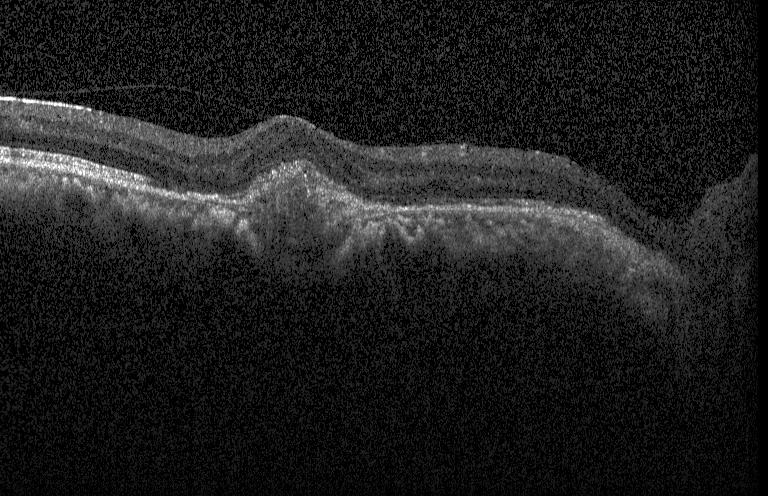

Diagnosis: choroidal neovascularization.